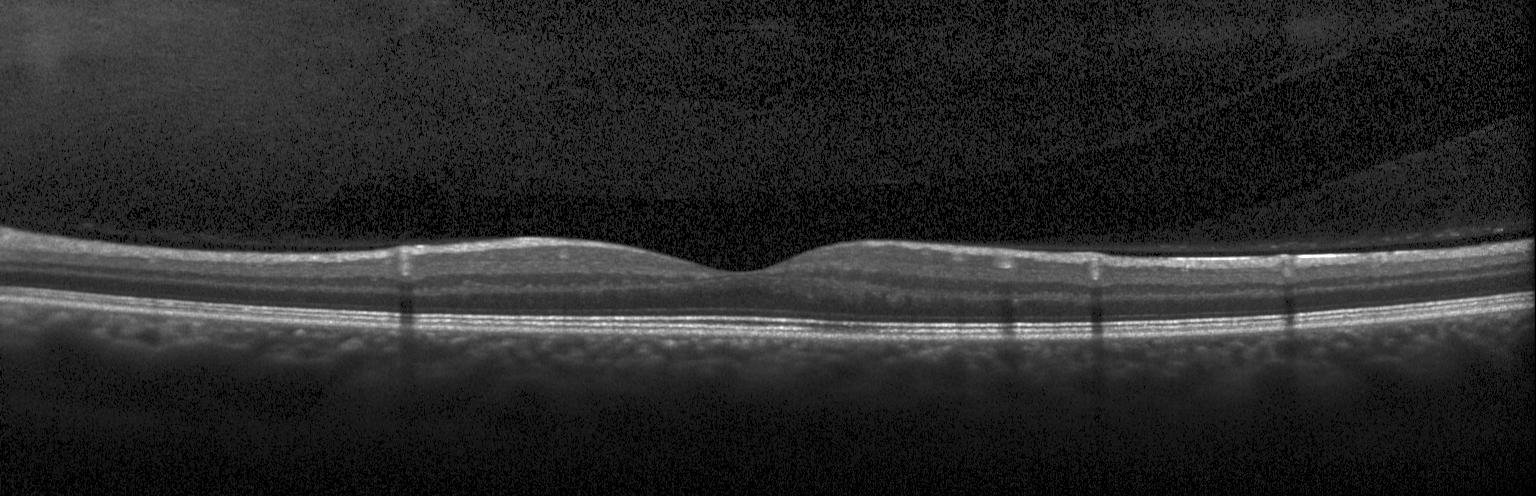 Optical coherence tomography scan.
Diagnosis: neither choroidal neovascularization, diabetic macular edema, nor drusen.